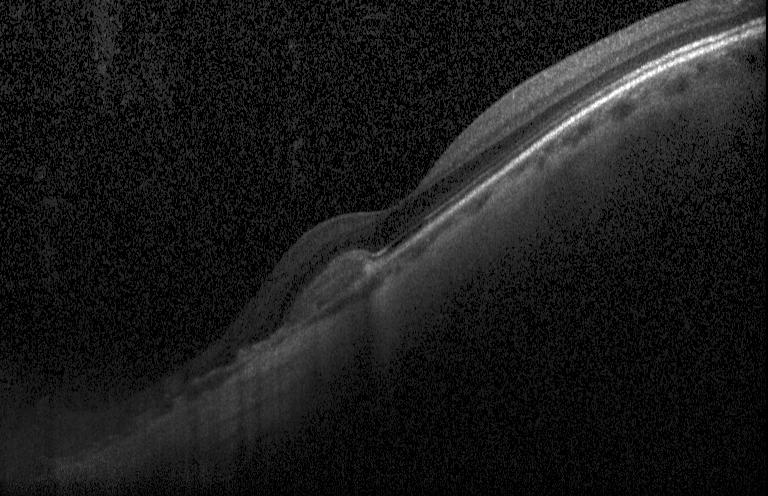
OCT finding: a choroidal neovascular membrane.